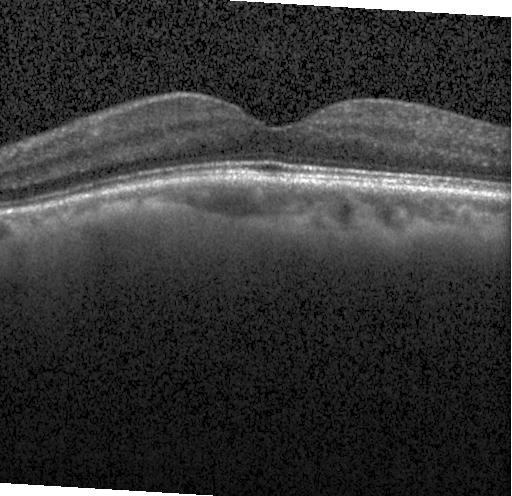 Macular scan · optical coherence tomography B-scan · Heidelberg Spectralis OCT system · spectral-domain OCT. This B-scan demonstrates no CNV, no DME, and no drusen.